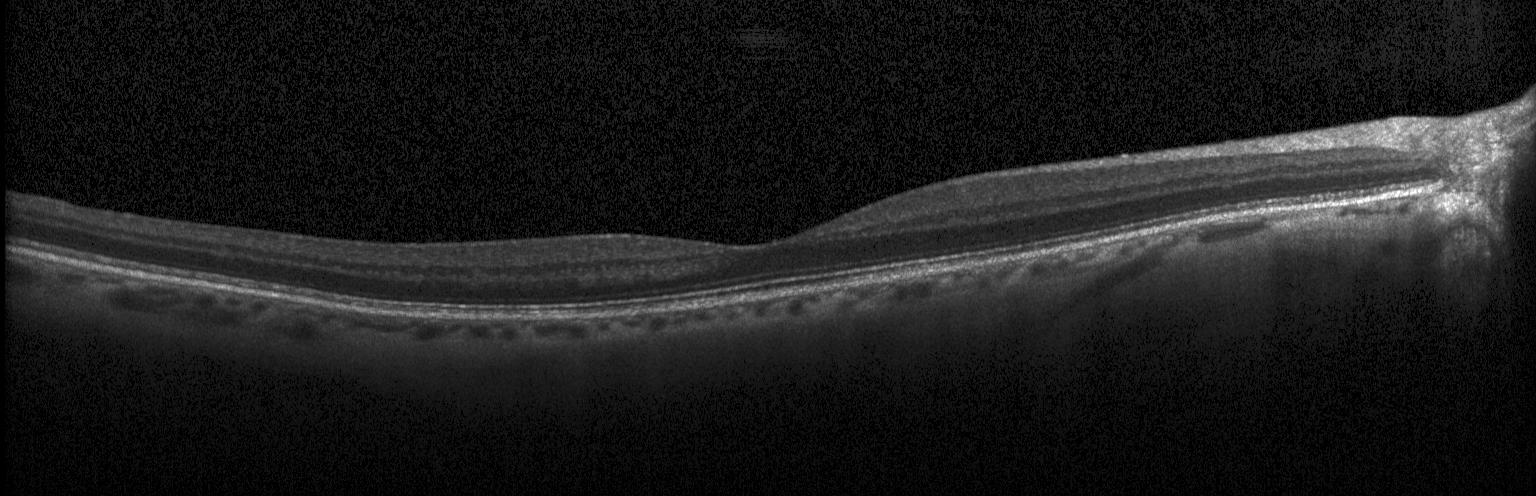 Heidelberg Spectralis OCT system; spectral-domain OCT; retinal OCT cross-section — Diagnosis: no evidence of CNV, DME, or drusen.